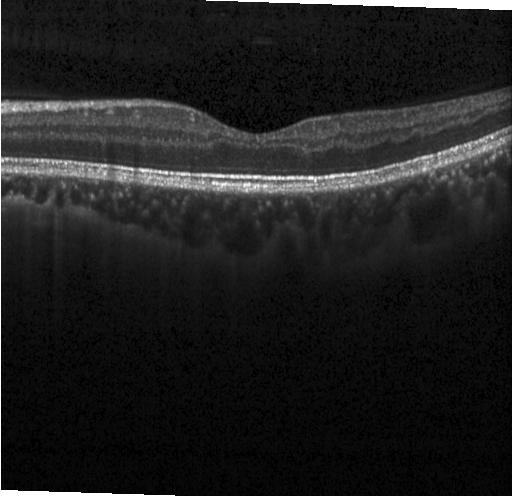
Retinal OCT cross-section showing neither choroidal neovascularization, diabetic macular edema, nor drusen.